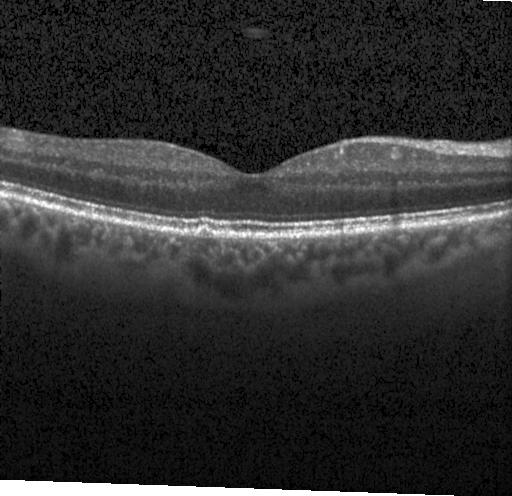
Centered on the fovea. Heidelberg Spectralis. SD-OCT. Retinal OCT B-scan.
Impression: sub-RPE drusenoid deposits.